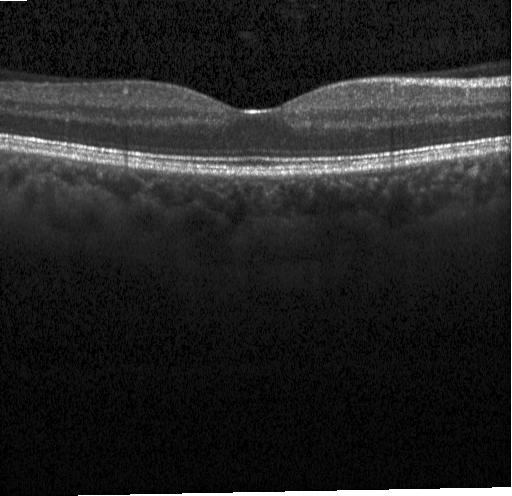 No CNV, DME, or drusen.